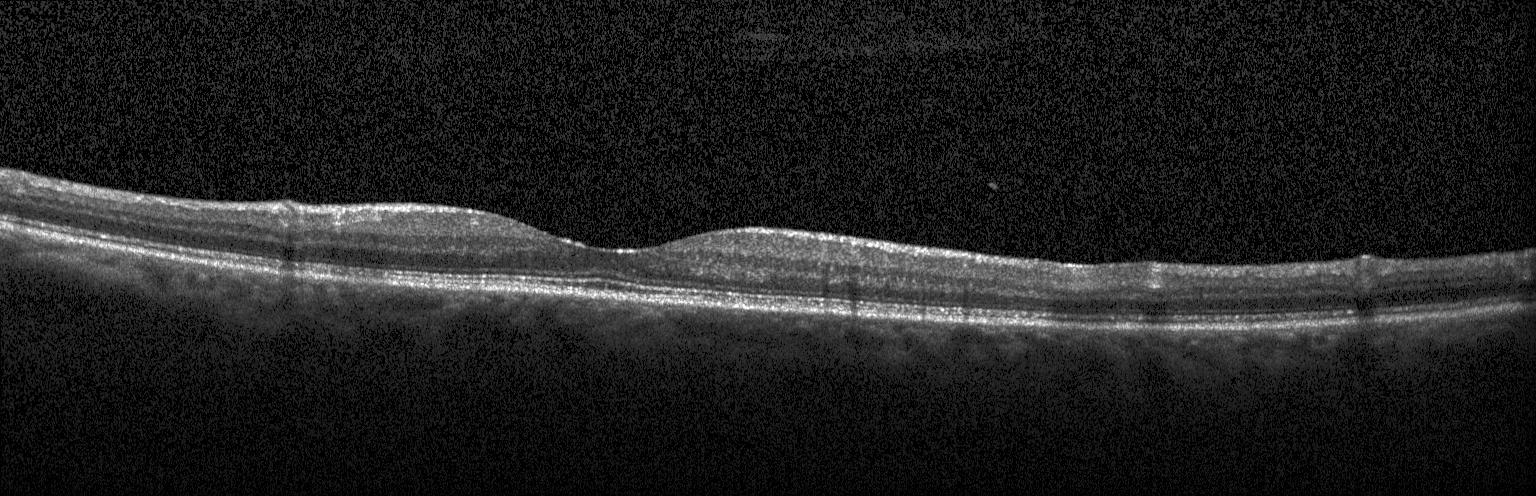

Optical coherence tomography scan.
This B-scan demonstrates no choroidal neovascularization, diabetic macular edema, or drusen.